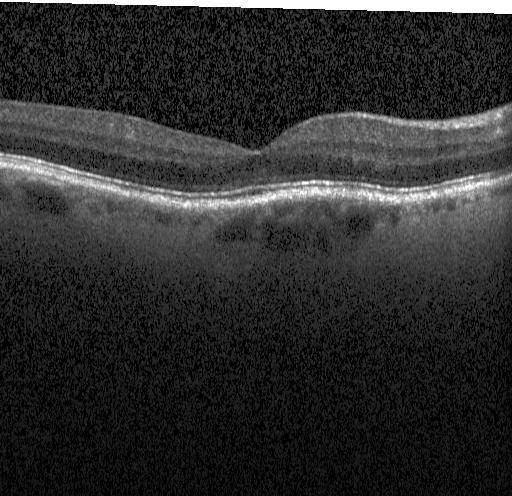

Optical coherence tomography scan; spectral-domain OCT; Heidelberg Spectralis; horizontal scan through the fovea.
Assessment: no evidence of CNV, DME, or drusen.